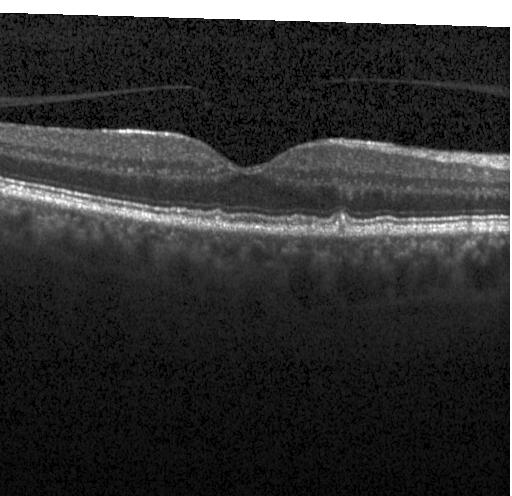 Retinal OCT cross-section, spectral-domain optical coherence tomography, horizontal scan through the fovea — OCT finding: multiple drusen.